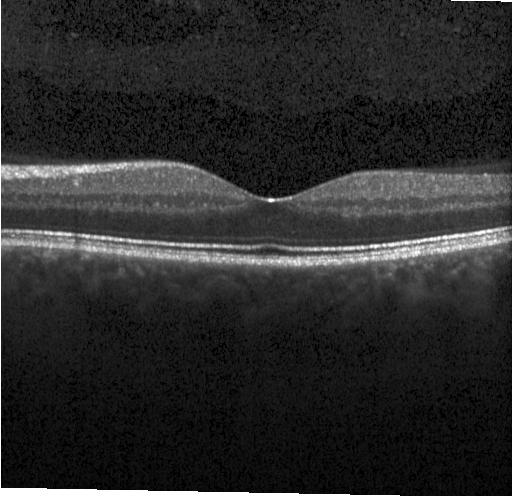

Heidelberg Spectralis OCT system. Retinal OCT B-scan. Assessment: no choroidal neovascularization, diabetic macular edema, or drusen.